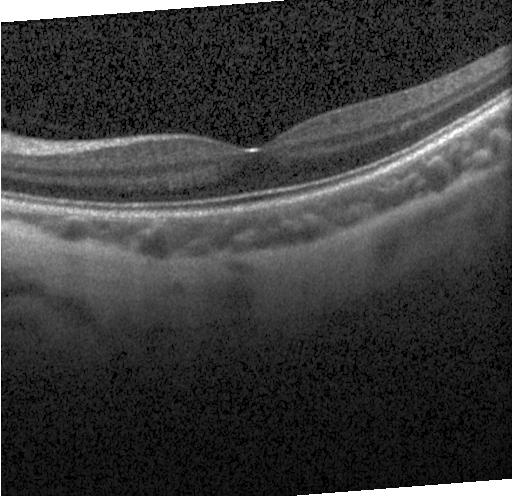
SD-OCT, OCT B-scan, macular scan, Heidelberg Spectralis
No choroidal neovascularization, no diabetic macular edema, and no drusen.